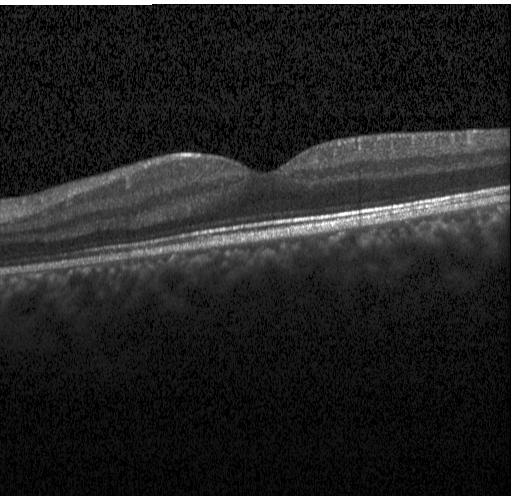 Retinal OCT B-scan, horizontal scan through the fovea, SD-OCT, instrument: Heidelberg Spectralis
Finding: no choroidal neovascularization, diabetic macular edema, or drusen.